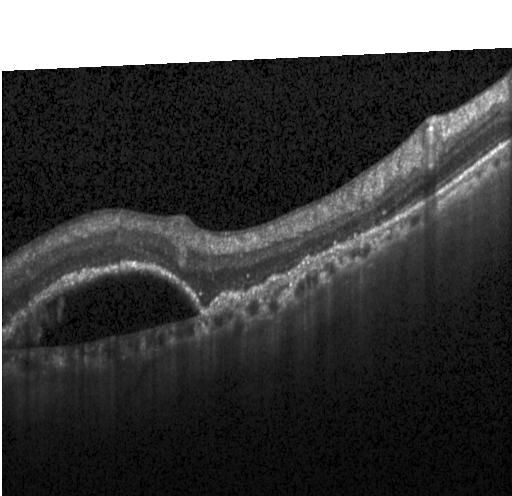
Fovea-centered, retinal OCT B-scan, SD-OCT, Heidelberg Spectralis OCT system. Diagnosis: CNV.